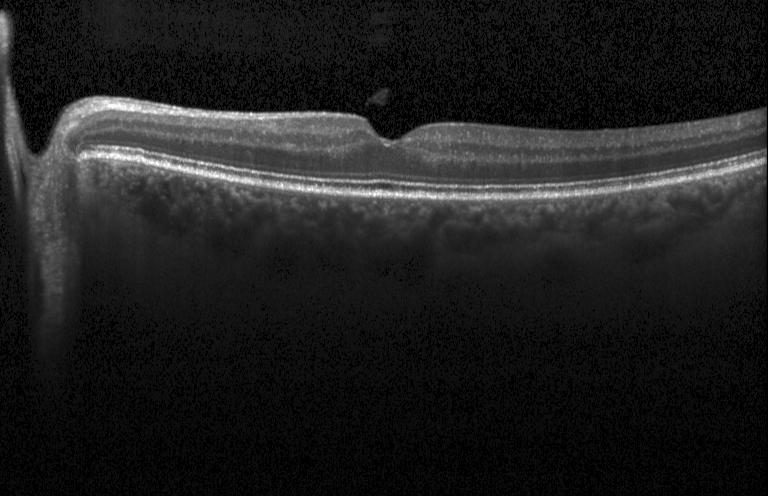
Spectral-domain OCT B-scan: neither CNV, DME, nor drusen.